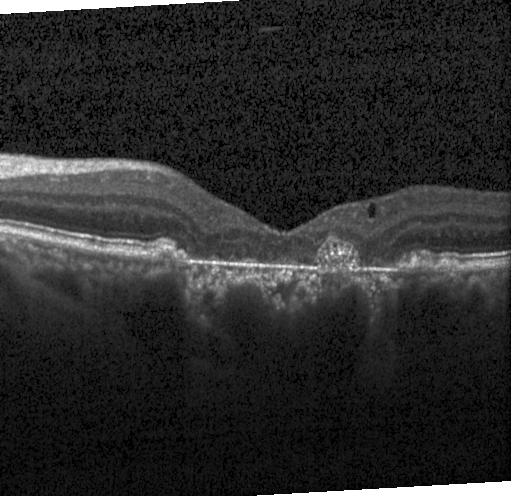 SD-OCT. Through the macula. Instrument: Heidelberg Spectralis. OCT B-scan — Finding: CNV.